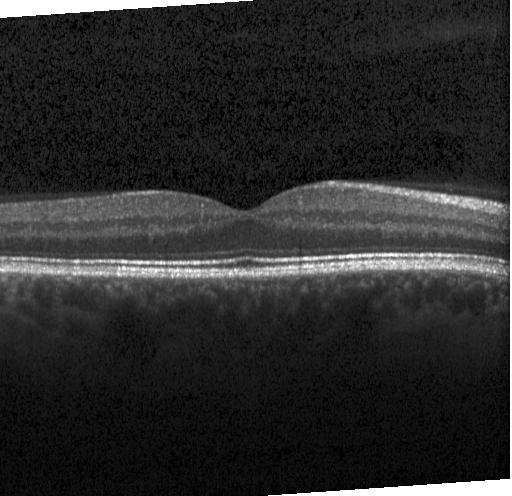

Dx: no choroidal neovascularization, no diabetic macular edema, and no drusen.